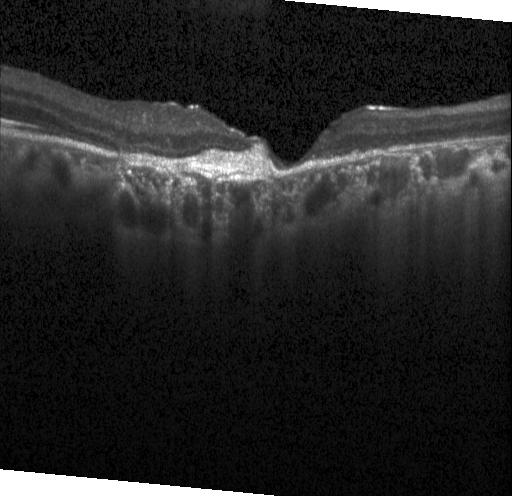 Retinal OCT cross-section. The scan shows CNV.